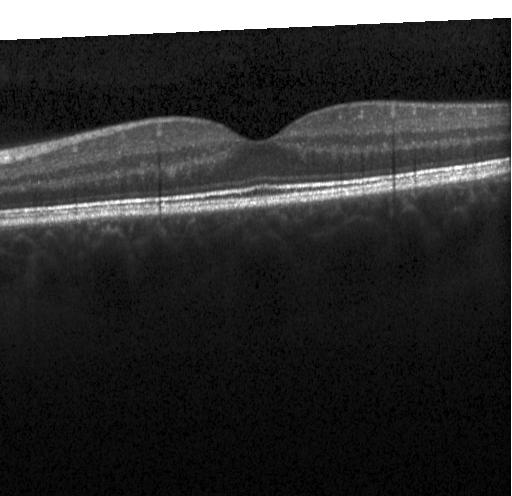

Diagnosis: no CNV, DME, or drusen.